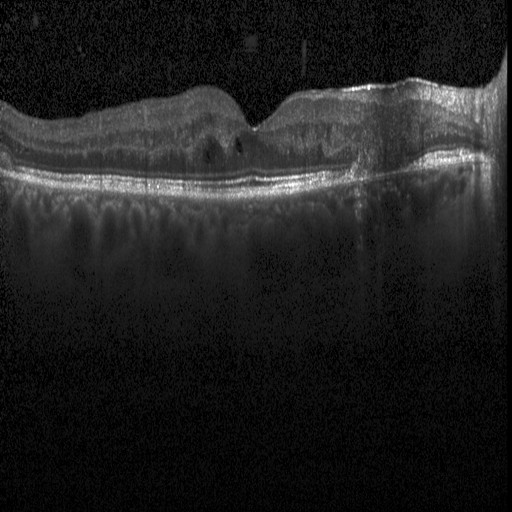

Spectral-domain OCT; Heidelberg Spectralis; retinal OCT B-scan — Macular OCT: DME.